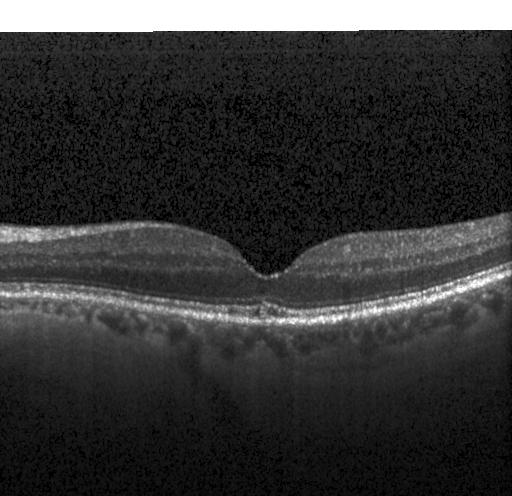

Spectral-domain OCT · optical coherence tomography B-scan — Diagnosis: neither CNV, DME, nor drusen.